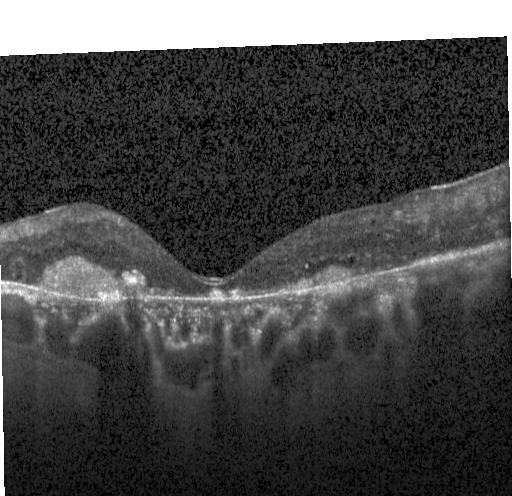

Spectral-domain OCT B-scan: a choroidal neovascular membrane.